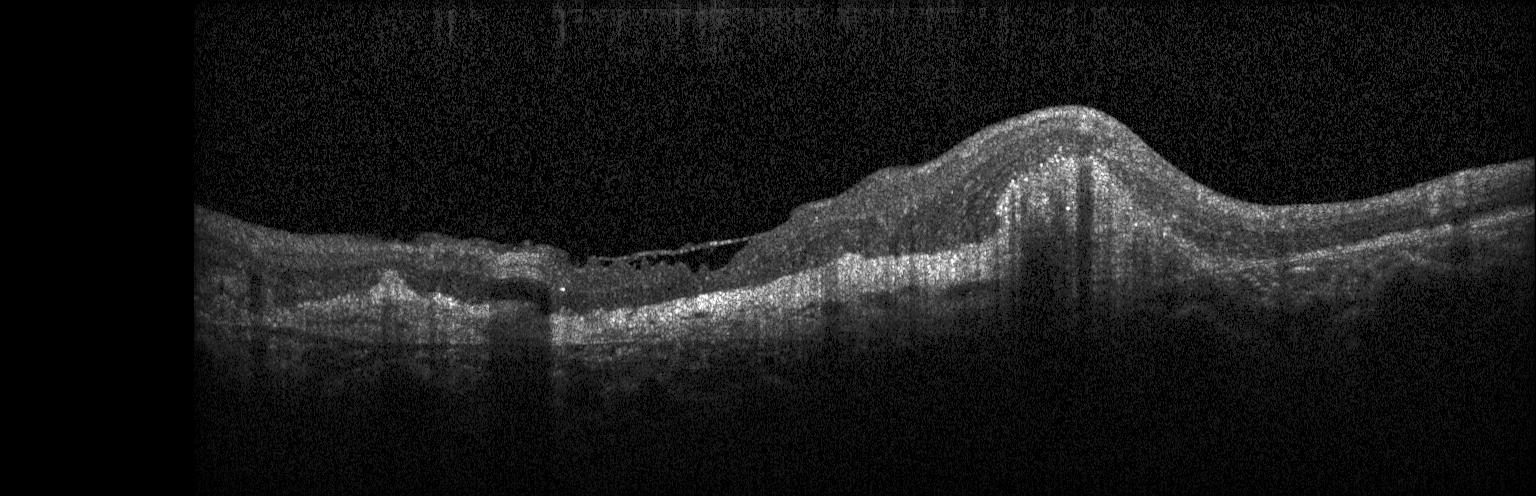
OCT finding: CNV.